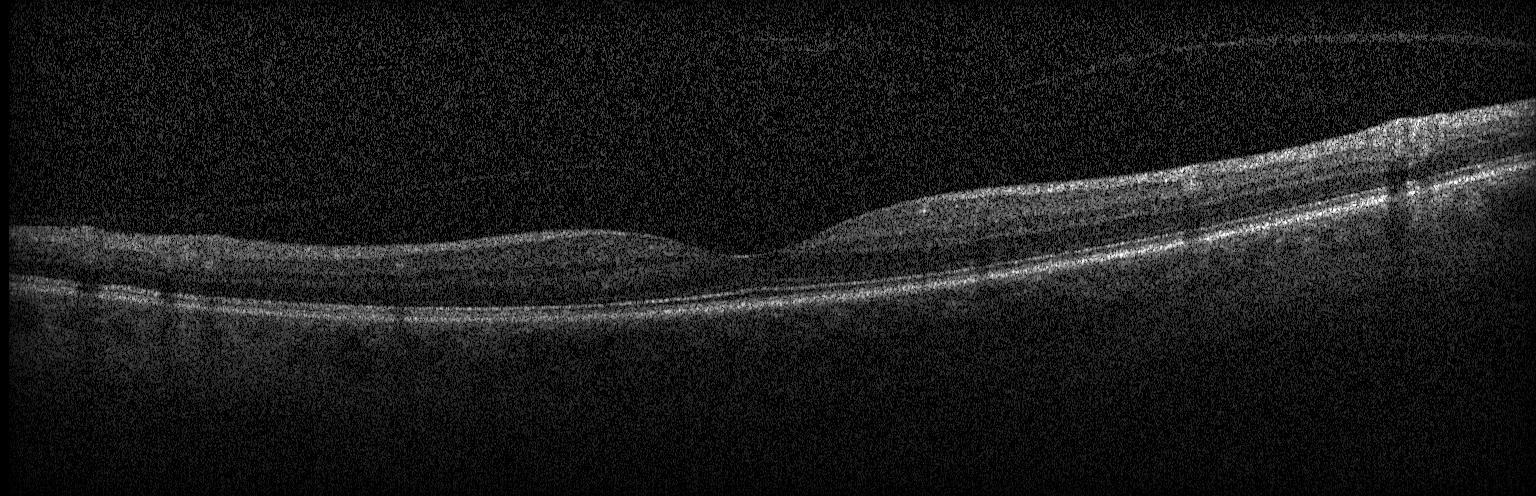
Macular OCT demonstrating no CNV, DME, or drusen.